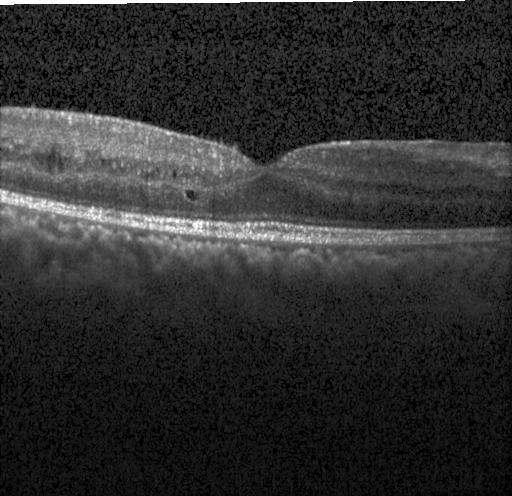 Macular OCT demonstrating DME.